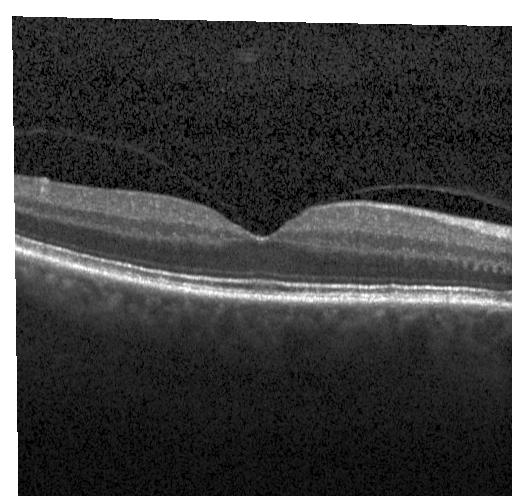 OCT B-scan — OCT finding: no evidence of choroidal neovascularization, diabetic macular edema, or drusen.